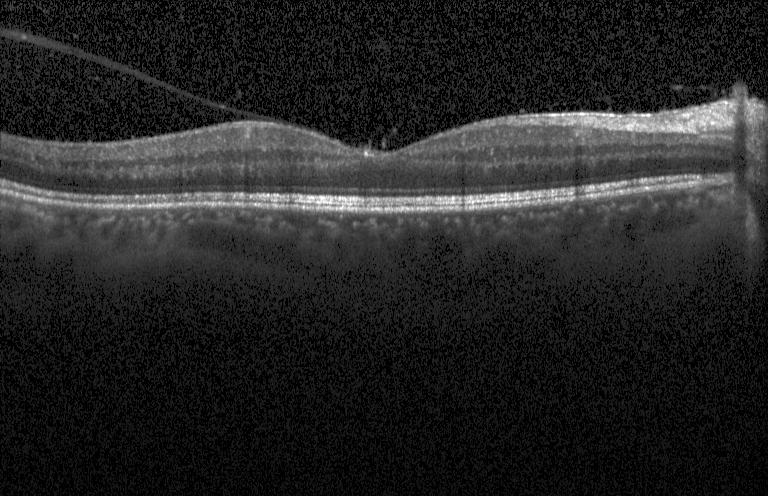 Assessment: neither CNV, DME, nor drusen.